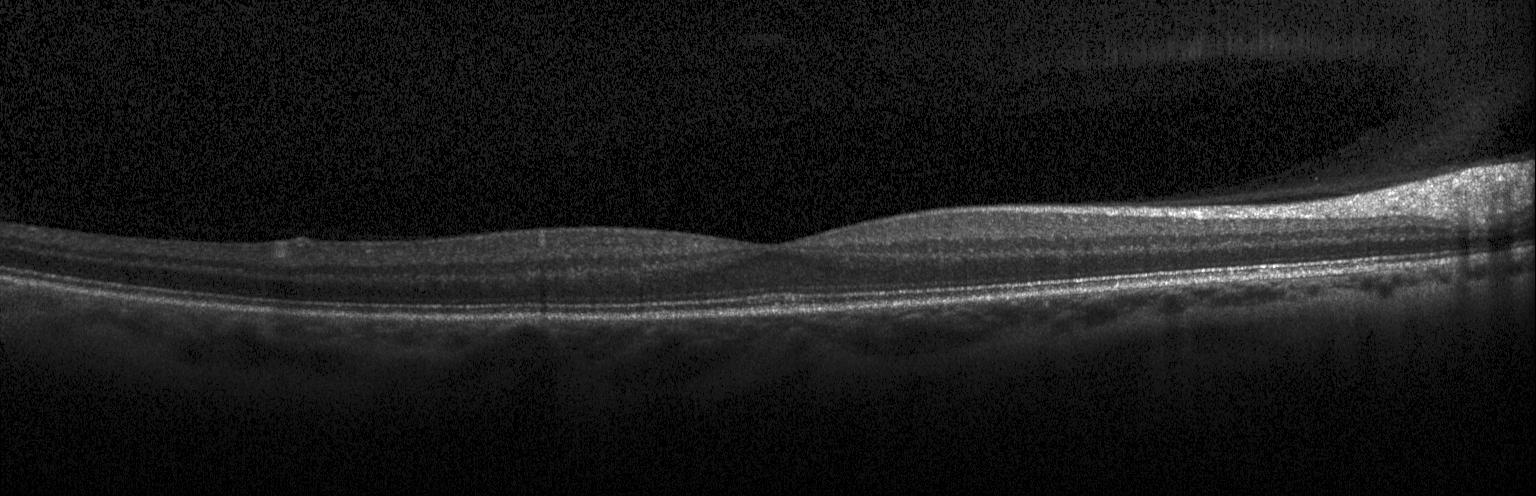 The scan shows neither choroidal neovascularization, diabetic macular edema, nor drusen.